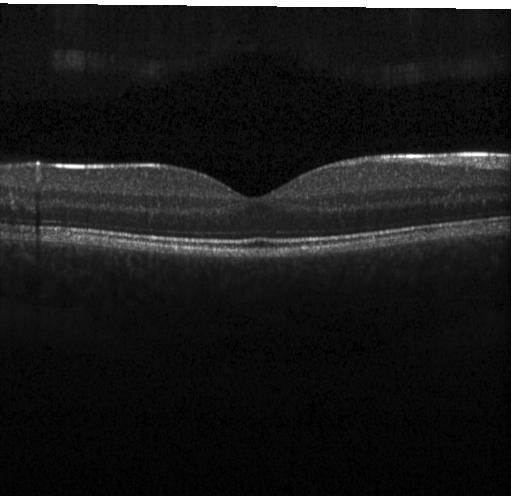
Optical coherence tomography scan
This B-scan demonstrates neither choroidal neovascularization, diabetic macular edema, nor drusen.